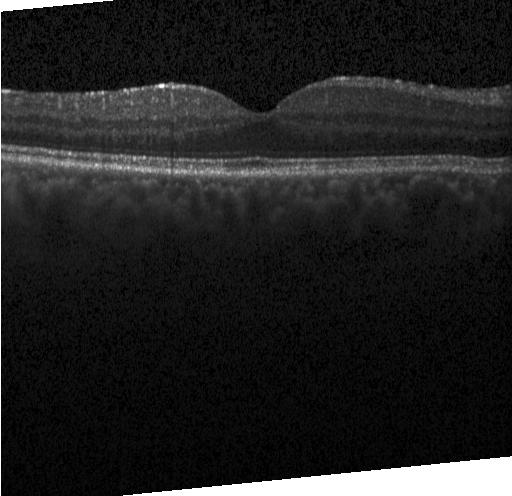

Spectral-domain optical coherence tomography, Heidelberg Spectralis, centered on the fovea, retinal OCT cross-section.
Dx: no CNV, DME, or drusen.